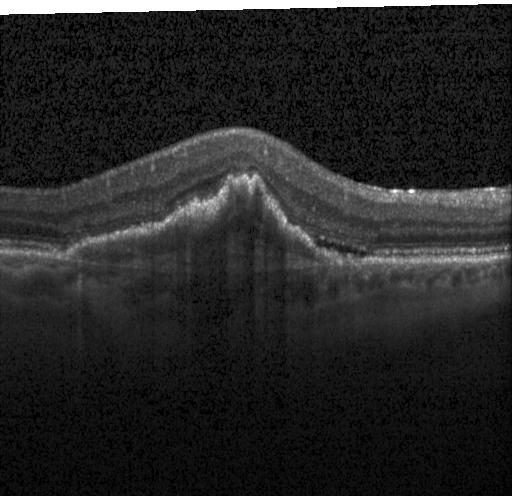

OCT finding: choroidal neovascularization.